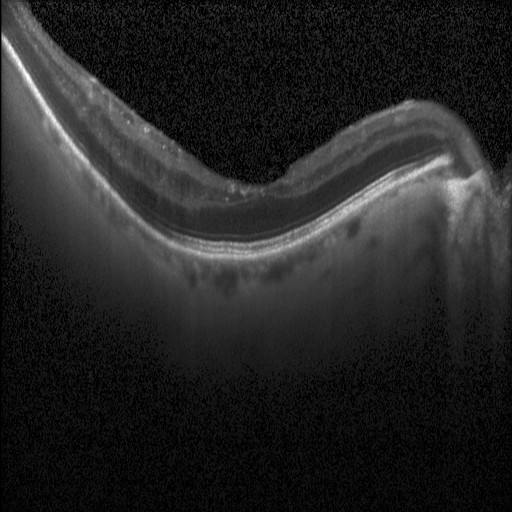

OCT line scan.
Diagnosis: diabetic macular edema (DME).